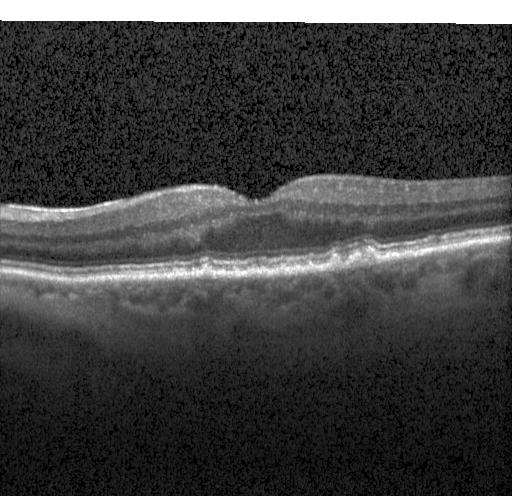

Macular scan. OCT line scan. Macular OCT: sub-RPE drusenoid deposits.